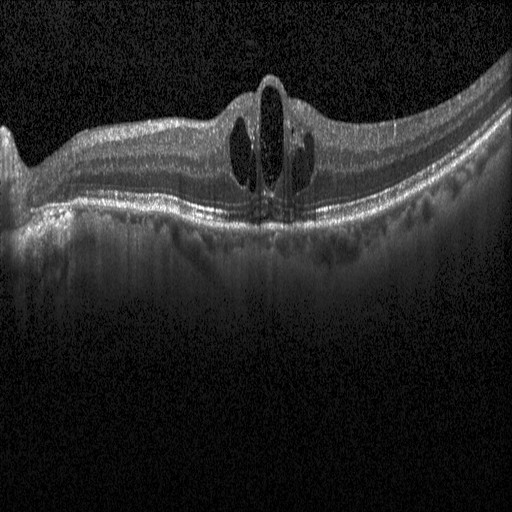

Through the macula. OCT line scan. Spectral-domain optical coherence tomography
Dx: diabetic macular edema (DME).